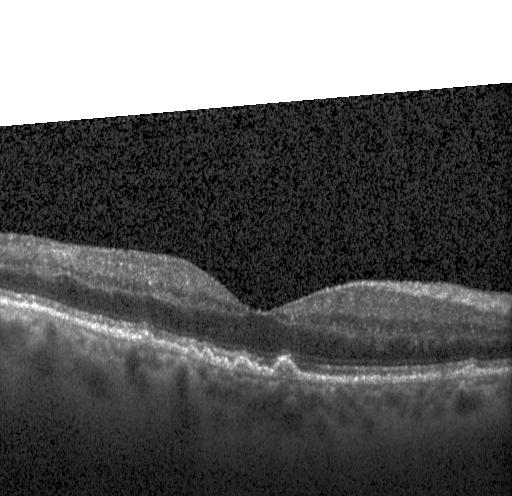 OCT line scan · SD-OCT — Drusen.